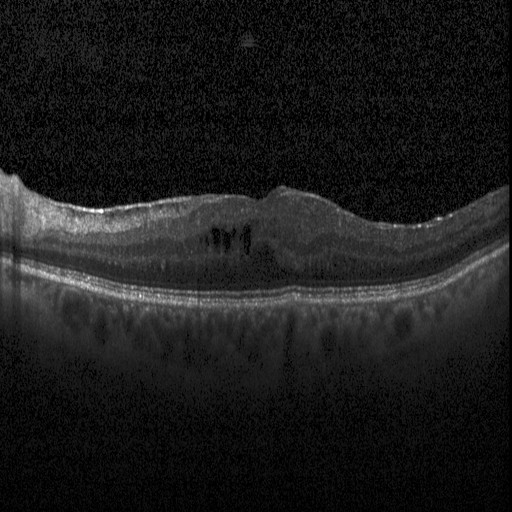
OCT finding: DME.